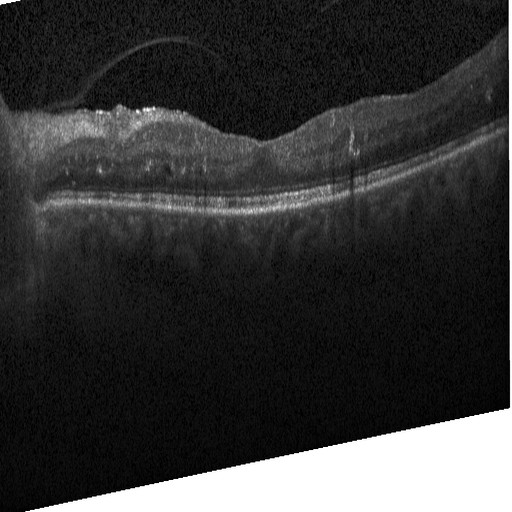 Heidelberg Spectralis OCT system. OCT line scan. Through the macula. SD-OCT
Assessment: DME.